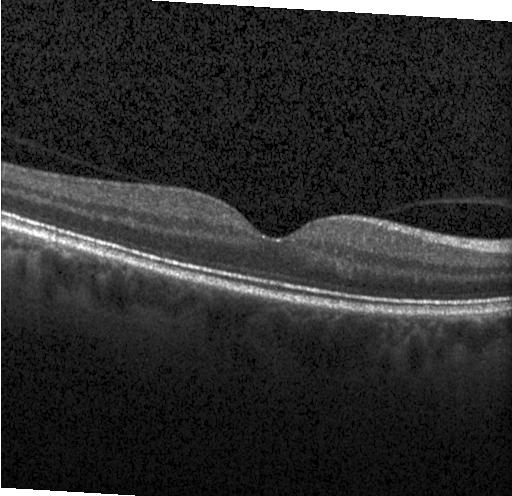

Through the macula. Spectral-domain OCT. Optical coherence tomography B-scan. Heidelberg Spectralis.
Finding: no CNV, DME, or drusen.